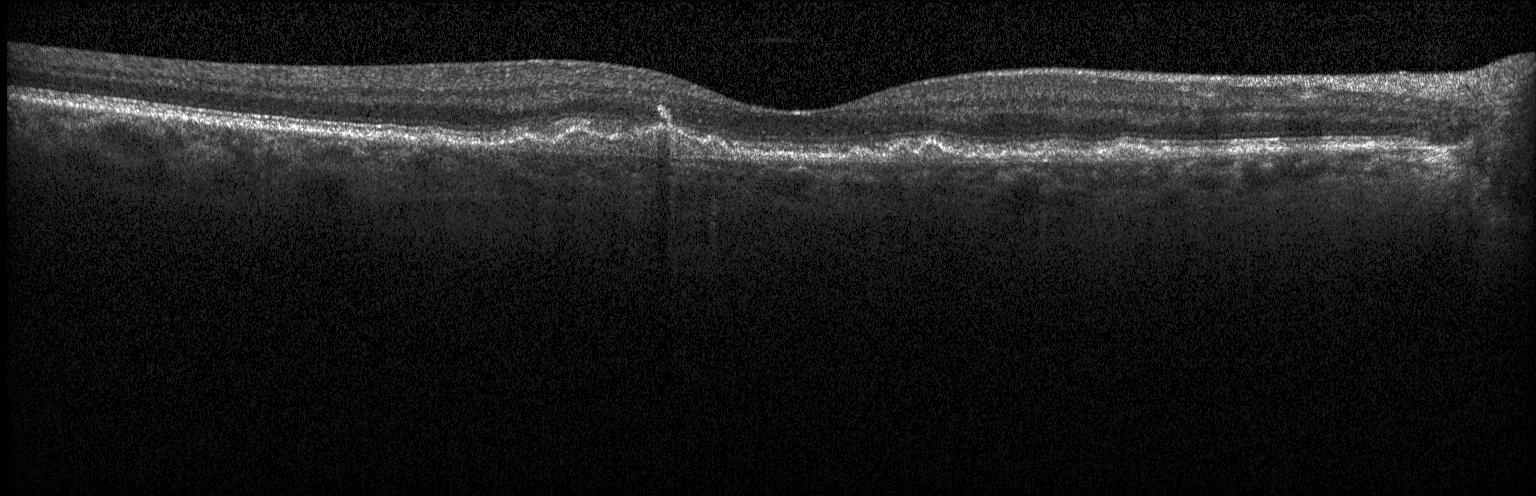

Retinal OCT cross-section showing CNV.